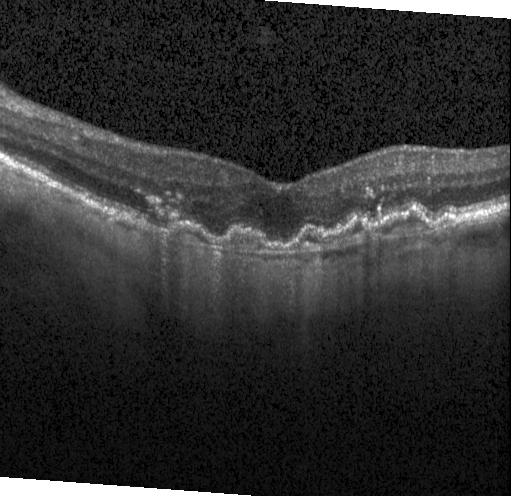 Macular OCT: choroidal neovascularization.